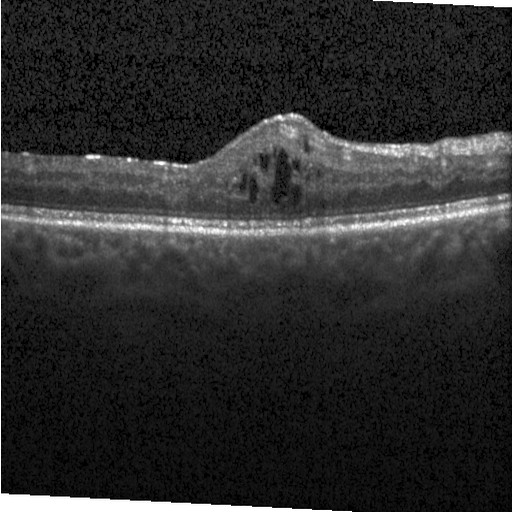
Heidelberg Spectralis OCT system. Optical coherence tomography B-scan — OCT finding: diabetic macular edema (DME).